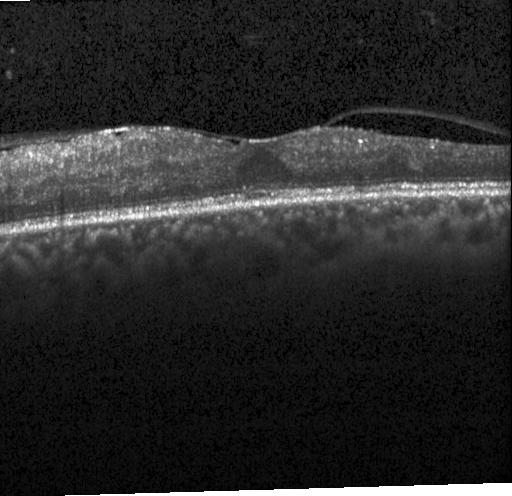
OCT finding: diabetic macular edema.